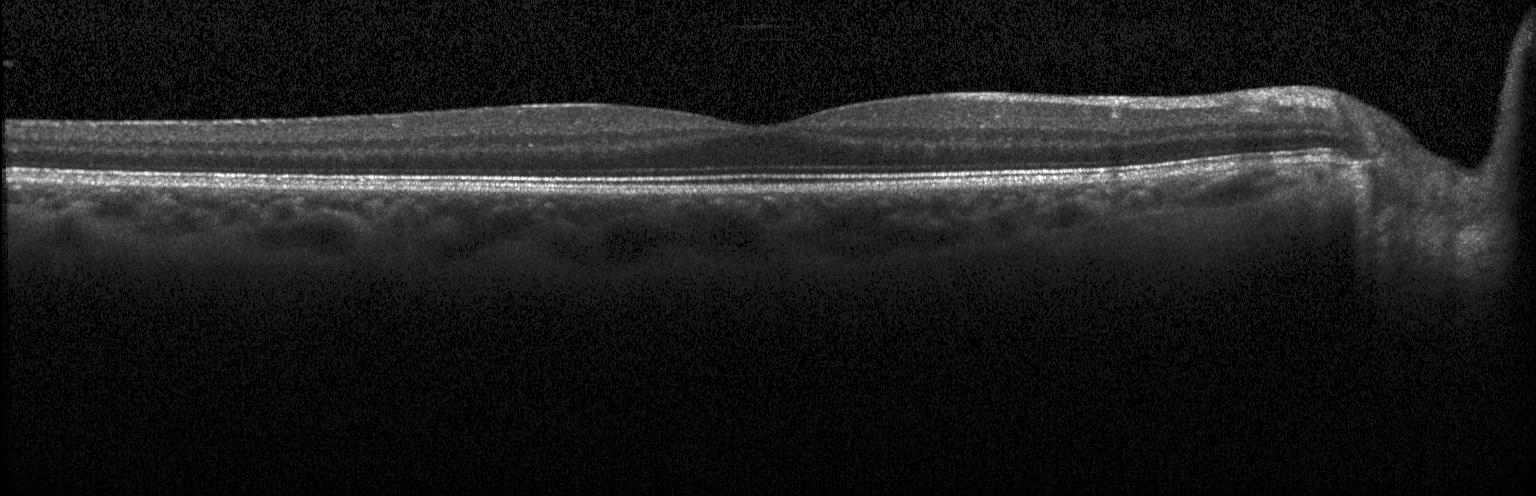
Heidelberg Spectralis · optical coherence tomography B-scan · centered on the fovea · SD-OCT — OCT finding: neither choroidal neovascularization, diabetic macular edema, nor drusen.